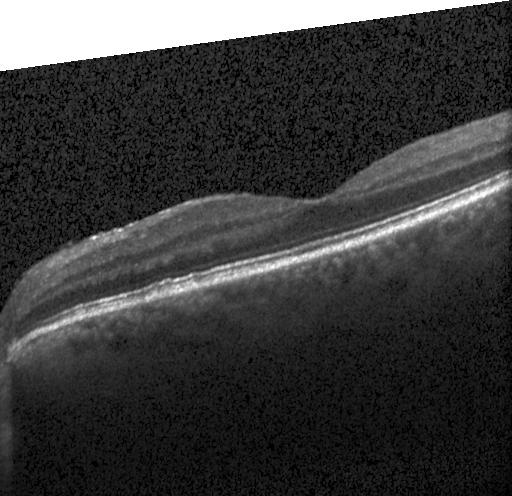
Optical coherence tomography B-scan — The scan shows neither choroidal neovascularization, diabetic macular edema, nor drusen.